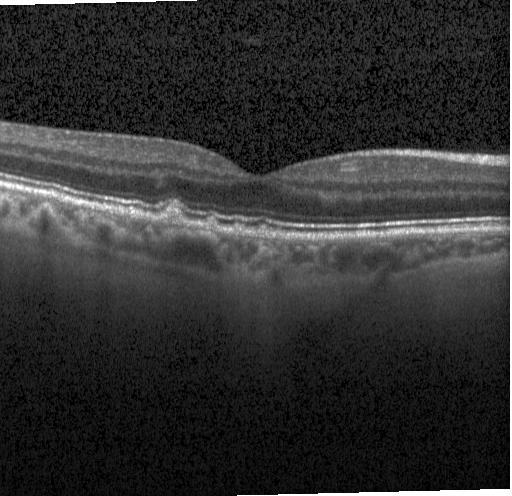
Optical coherence tomography scan; horizontal scan through the fovea
Impression: drusen.